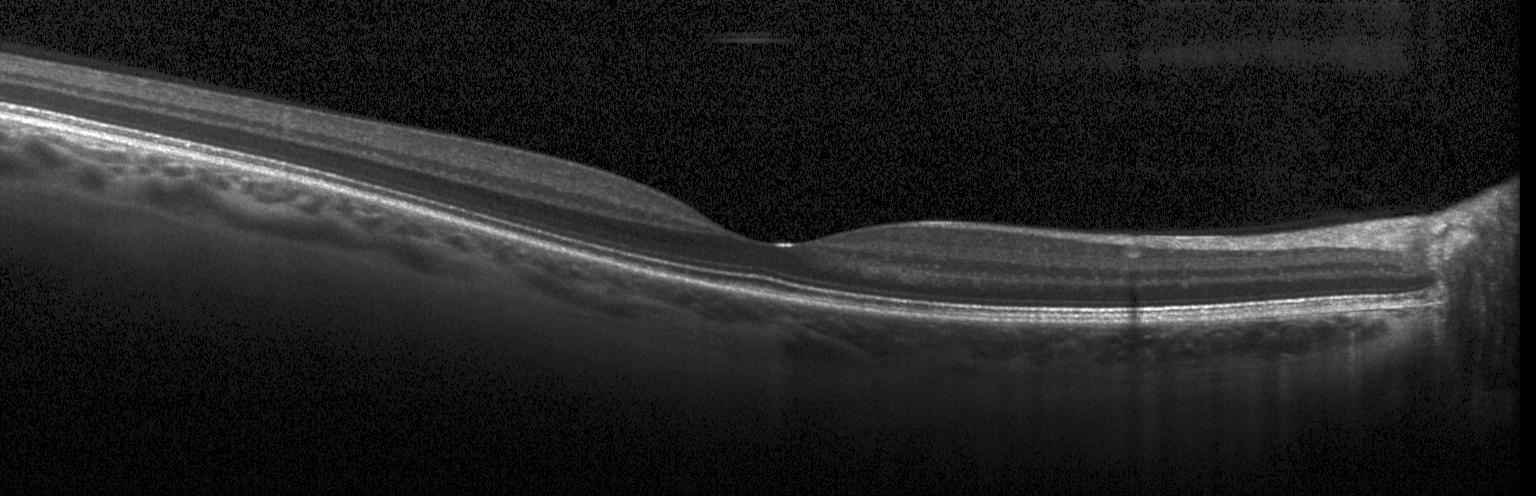 Instrument: Heidelberg Spectralis. OCT line scan. Fovea-centered
Impression: no CNV, DME, or drusen.